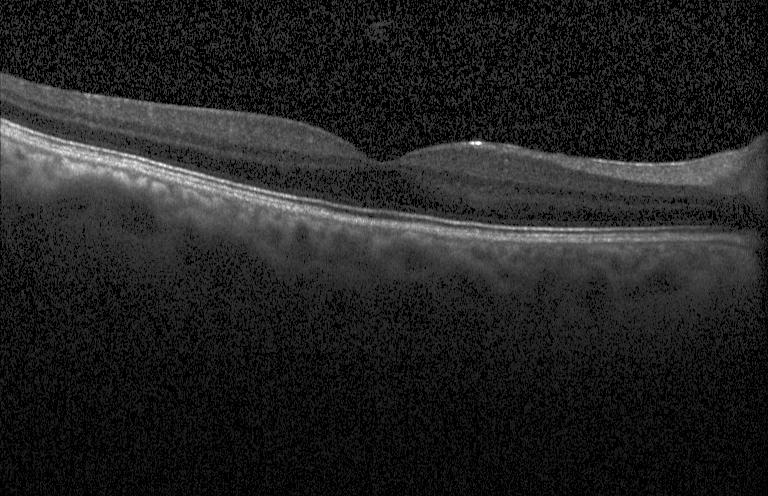 The scan shows no evidence of choroidal neovascularization, diabetic macular edema, or drusen.